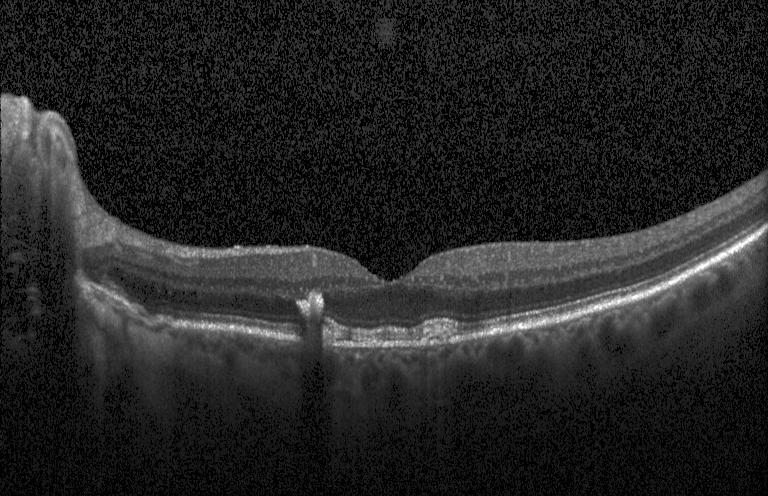
Optical coherence tomography B-scan; horizontal scan through the fovea; acquired on a Heidelberg Spectralis
Dx: sub-RPE drusenoid deposits.